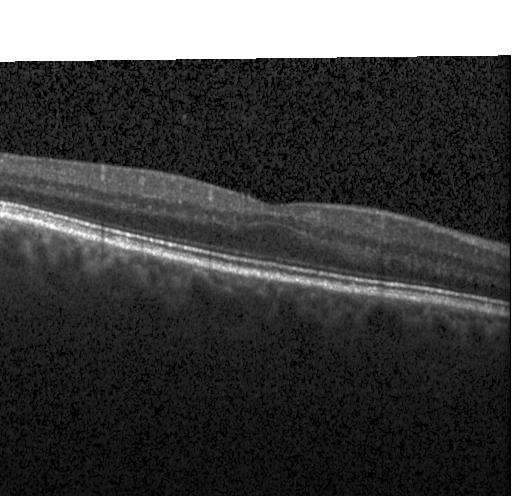

Macular OCT: no evidence of choroidal neovascularization, diabetic macular edema, or drusen.